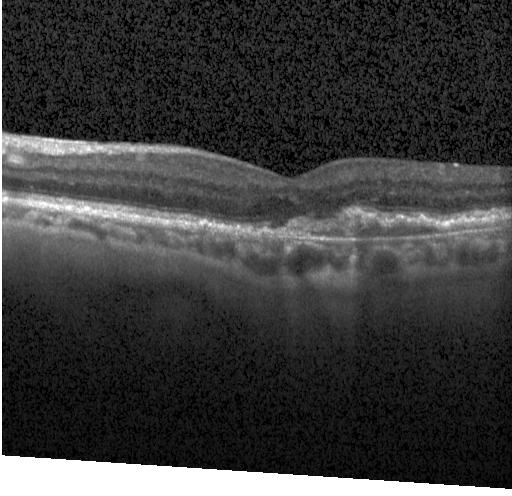
Impression: a choroidal neovascular membrane.